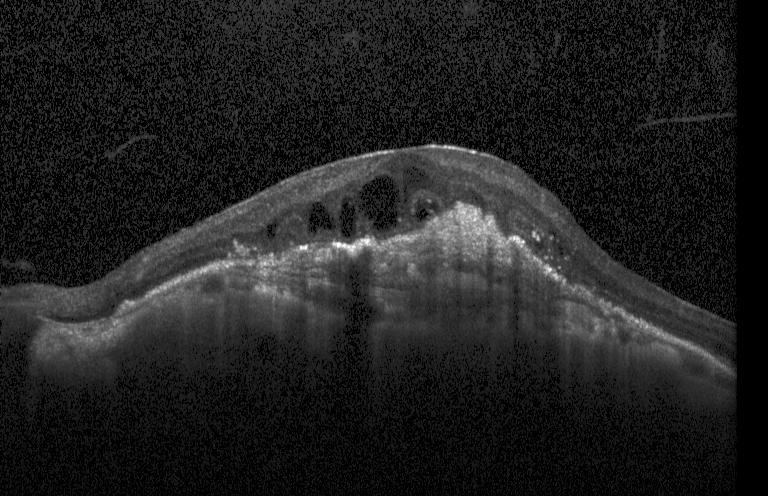

Finding: choroidal neovascularization (CNV).